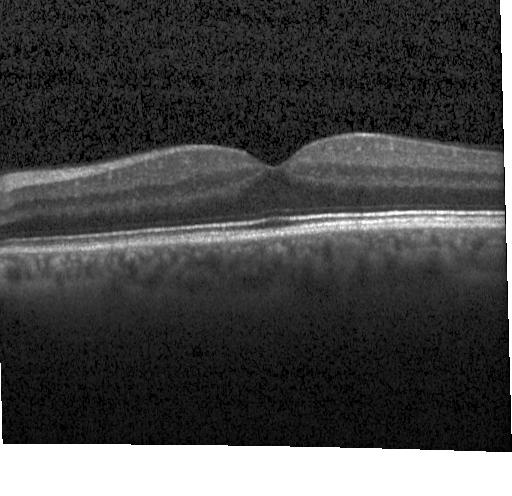
Optical coherence tomography B-scan. The scan shows no evidence of choroidal neovascularization, diabetic macular edema, or drusen.